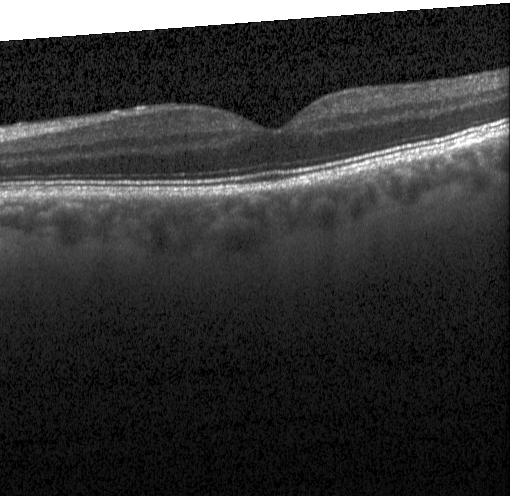 Assessment: neither choroidal neovascularization, diabetic macular edema, nor drusen.